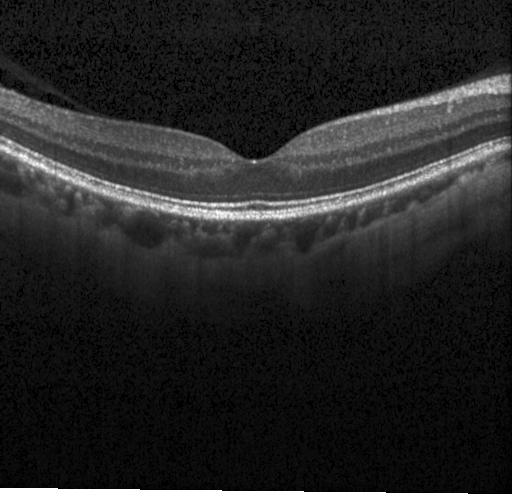 Retinal OCT cross-section, horizontal scan through the fovea, instrument: Heidelberg Spectralis — OCT finding: no CNV, no DME, and no drusen.